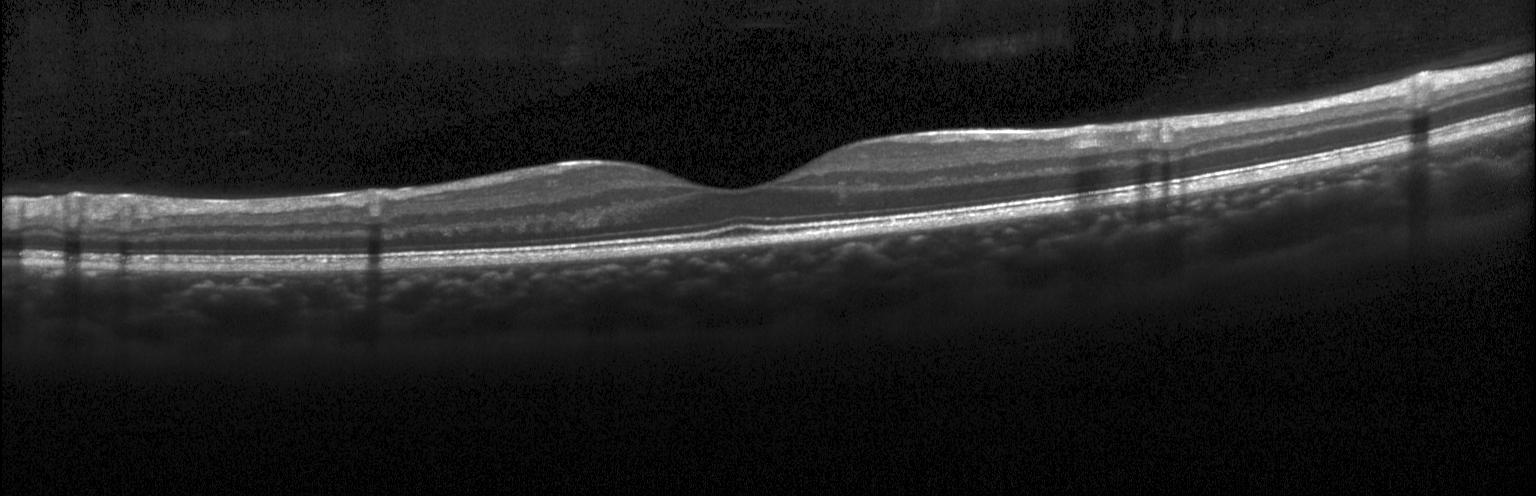

Diagnosis: no choroidal neovascularization, no diabetic macular edema, and no drusen.